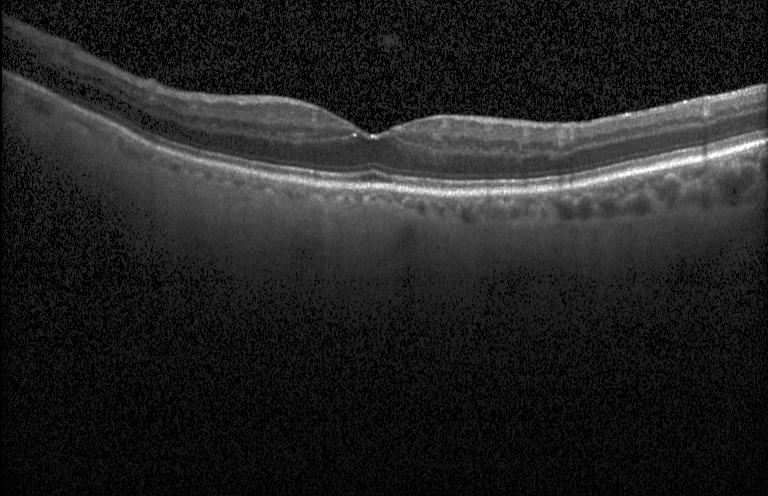 Acquired on a Heidelberg Spectralis; optical coherence tomography scan; horizontal scan through the fovea
OCT finding: no CNV, DME, or drusen.